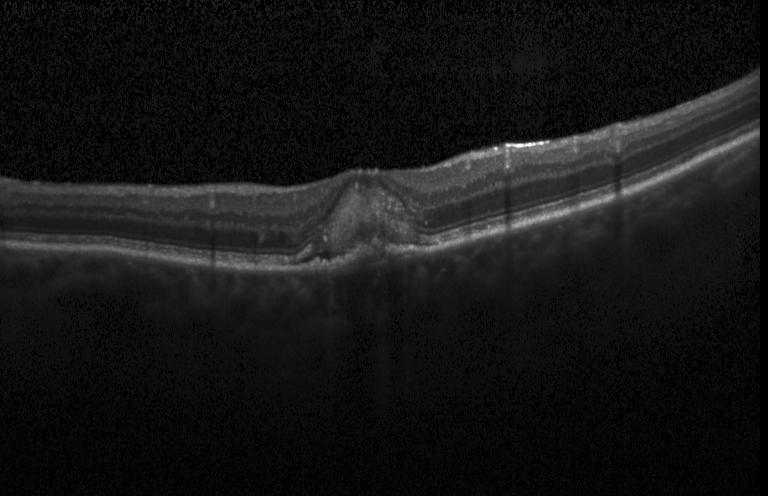 Diagnosis: a choroidal neovascular membrane.